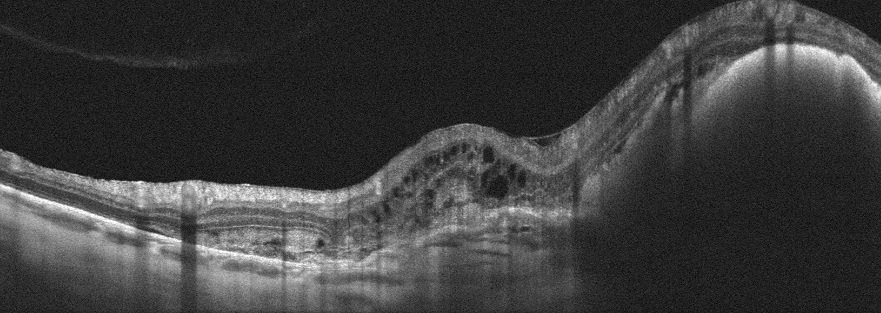 Optovue Avanti RTVue XR, macular scan, optical coherence tomography scan.
Finding: AMD.